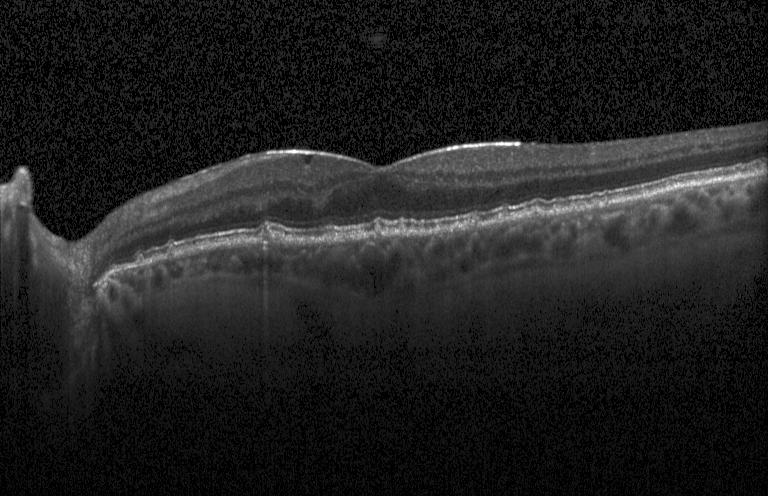 Macular scan, OCT B-scan, Heidelberg Spectralis. Finding: sub-RPE drusenoid deposits.